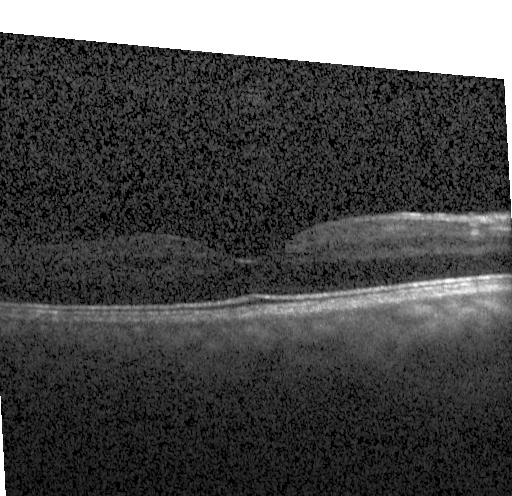 Centered on the fovea. Spectral-domain OCT. OCT line scan. Acquired on a Heidelberg Spectralis
Diagnosis: no choroidal neovascularization, diabetic macular edema, or drusen.